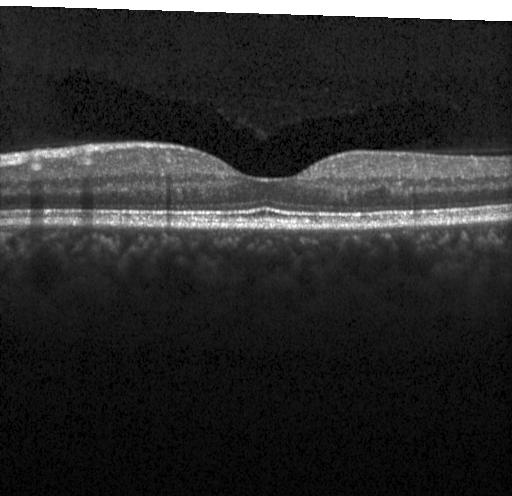
Diagnosis: no evidence of choroidal neovascularization, diabetic macular edema, or drusen.